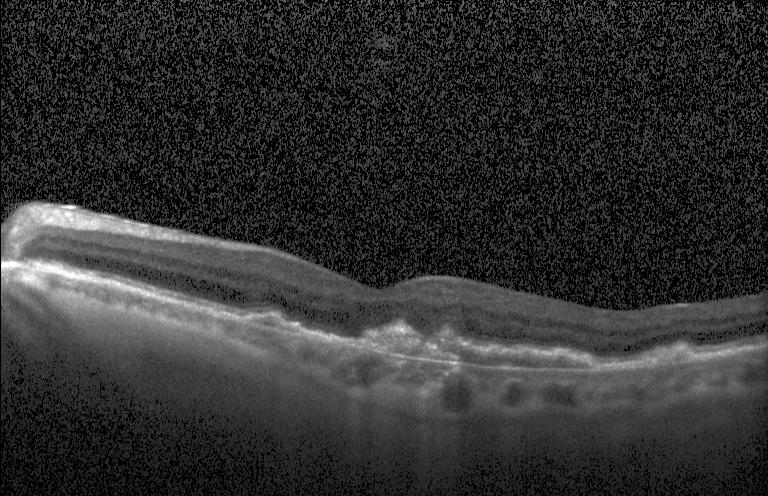
Optical coherence tomography B-scan
Impression: CNV.